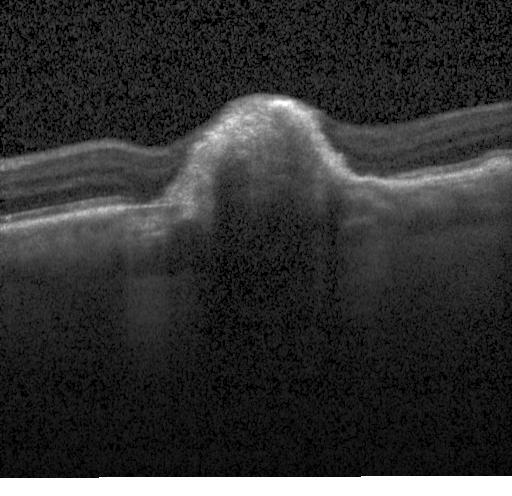 Instrument: Heidelberg Spectralis, centered on the fovea, OCT line scan. Impression: a choroidal neovascular membrane.